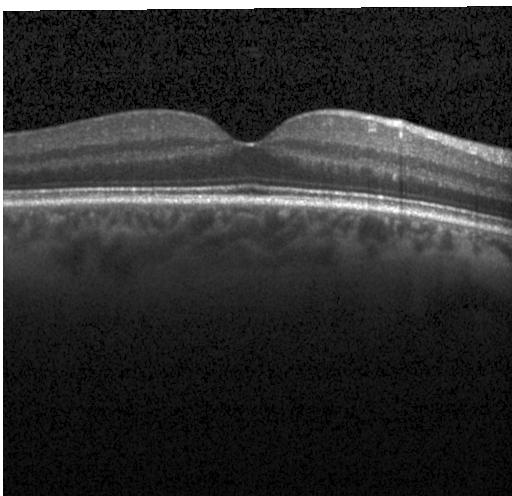 Macular scan. Retinal OCT cross-section
This B-scan demonstrates neither CNV, DME, nor drusen.